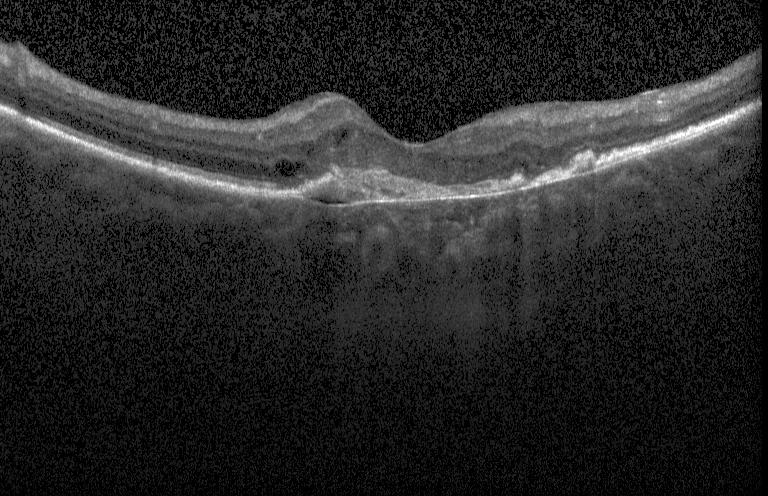
Heidelberg Spectralis OCT system · horizontal scan through the fovea · SD-OCT · retinal OCT B-scan. Finding: choroidal neovascularization (CNV).